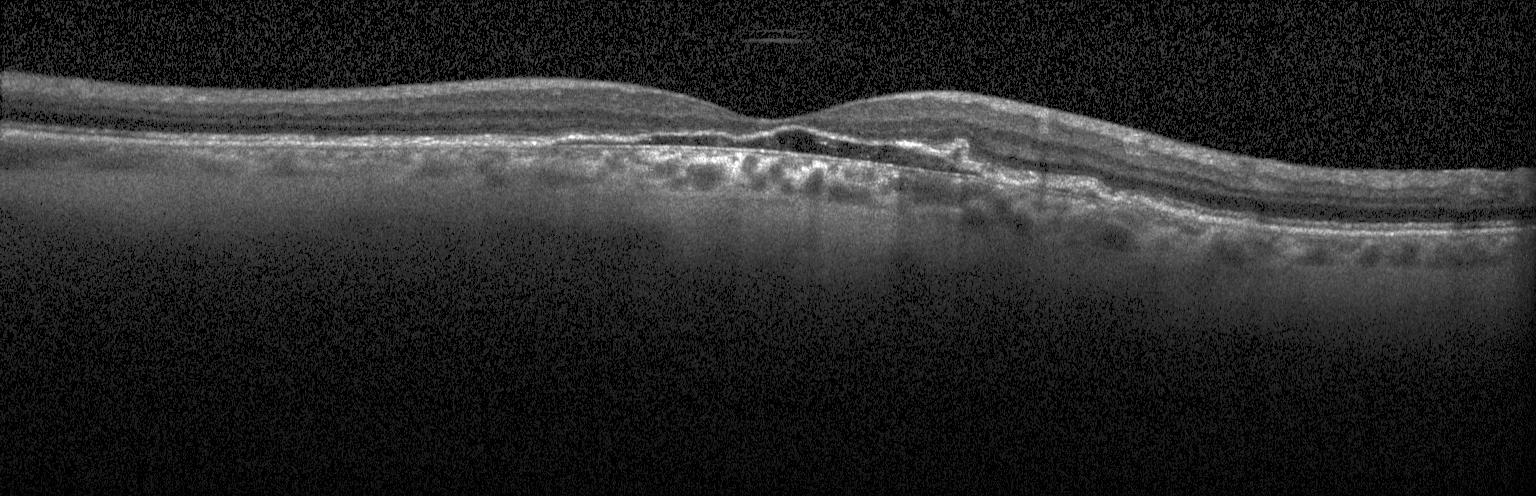

Heidelberg Spectralis OCT system, optical coherence tomography scan.
The scan shows a choroidal neovascular membrane.